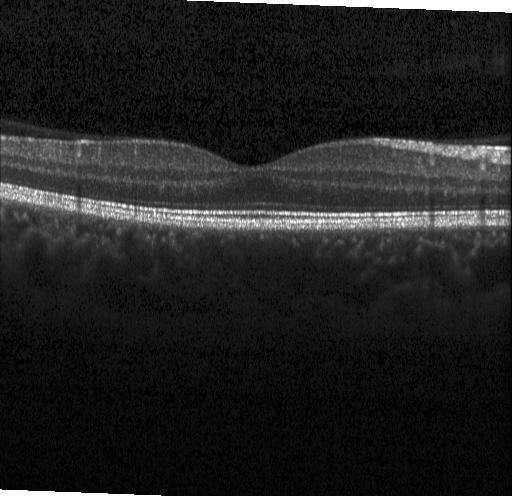
Retinal OCT cross-section showing no evidence of CNV, DME, or drusen.